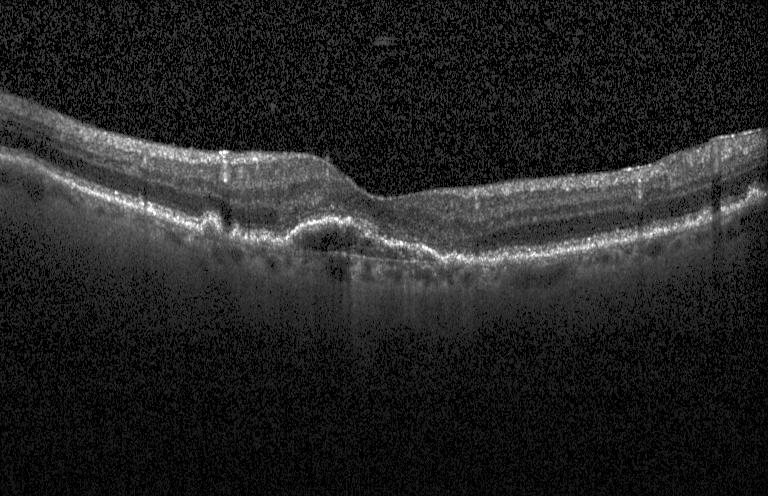

Optical coherence tomography scan, spectral-domain OCT, instrument: Heidelberg Spectralis, macular scan
OCT finding: choroidal neovascularization (CNV).